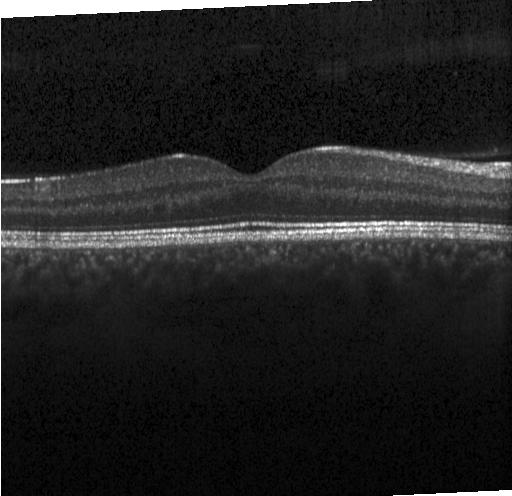

Retinal OCT cross-section. Heidelberg Spectralis OCT system — Assessment: no choroidal neovascularization, no diabetic macular edema, and no drusen.